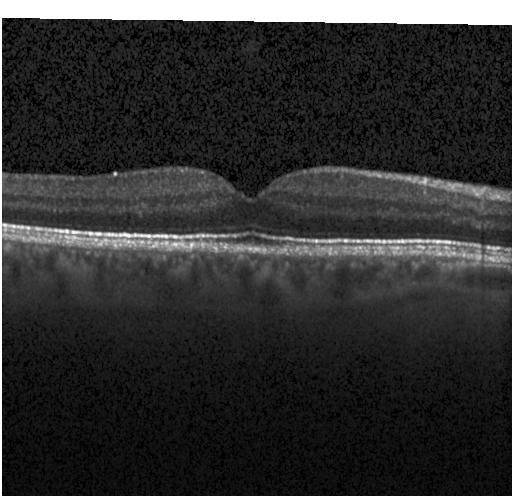
Instrument: Heidelberg Spectralis. Retinal OCT B-scan. Finding: no evidence of choroidal neovascularization, diabetic macular edema, or drusen.